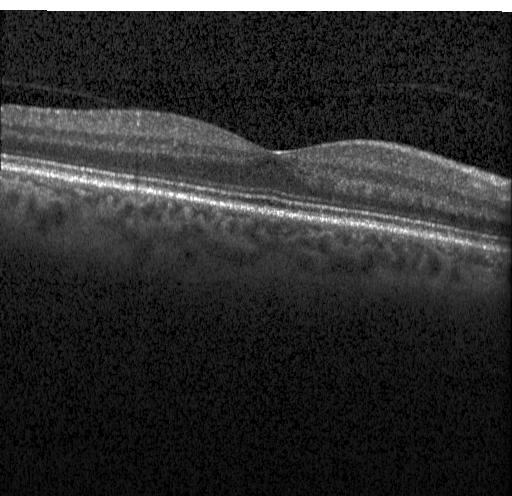

OCT B-scan showing no choroidal neovascularization, diabetic macular edema, or drusen.